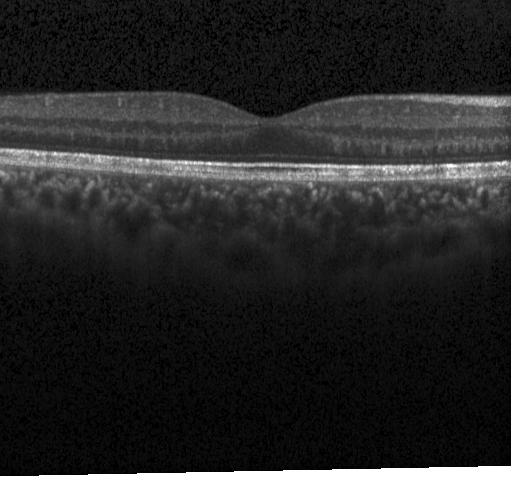

Impression: no choroidal neovascularization, diabetic macular edema, or drusen.